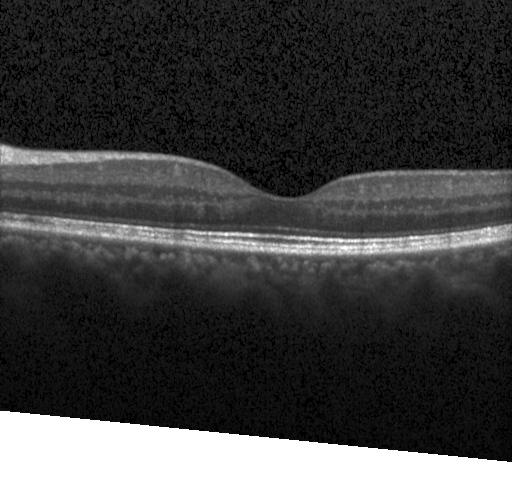

Optical coherence tomography scan; acquired on a Heidelberg Spectralis; spectral-domain optical coherence tomography; through the macula. Diagnosis: no choroidal neovascularization, no diabetic macular edema, and no drusen.